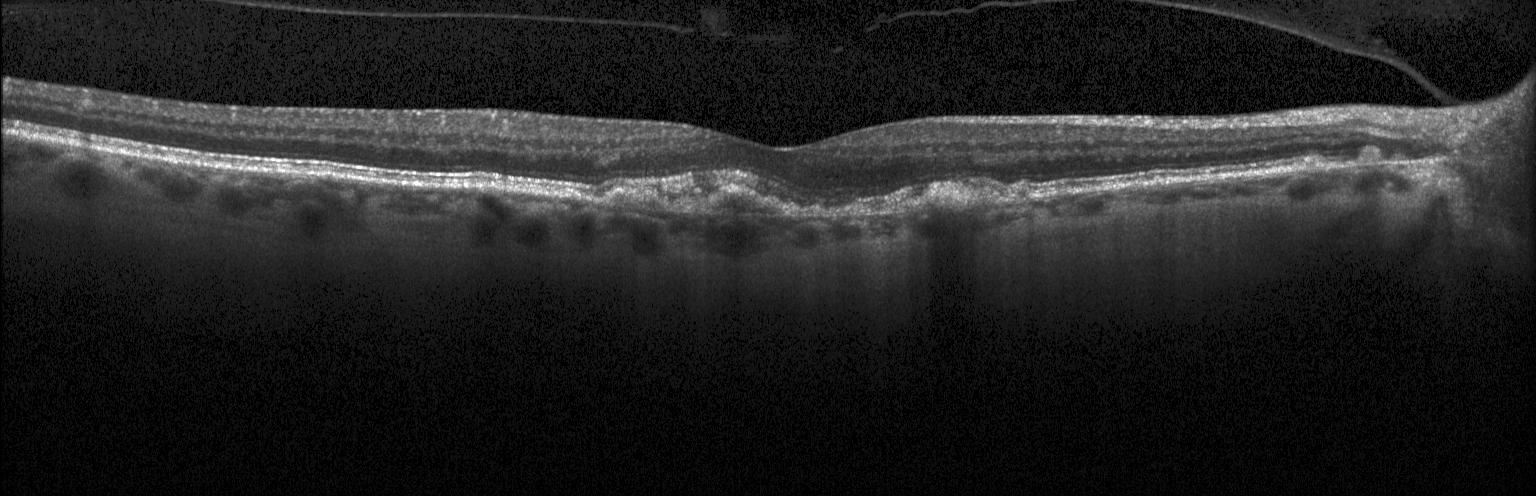 OCT line scan; spectral-domain OCT; instrument: Heidelberg Spectralis; fovea-centered. Impression: choroidal neovascularization.